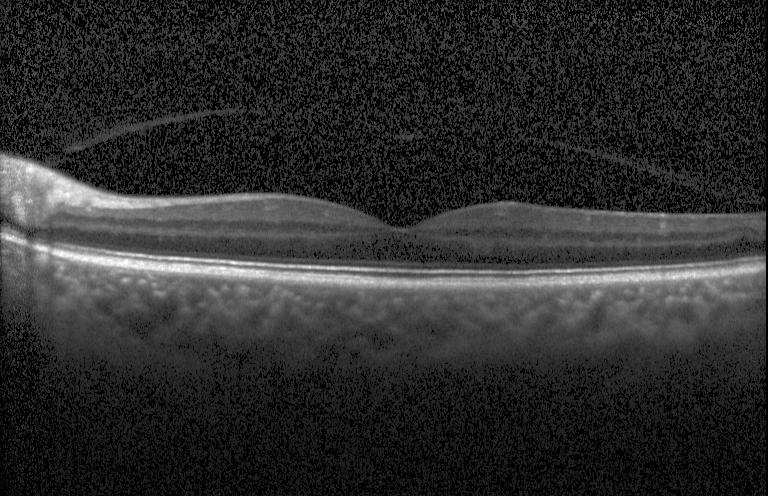 Diagnosis: no evidence of CNV, DME, or drusen.